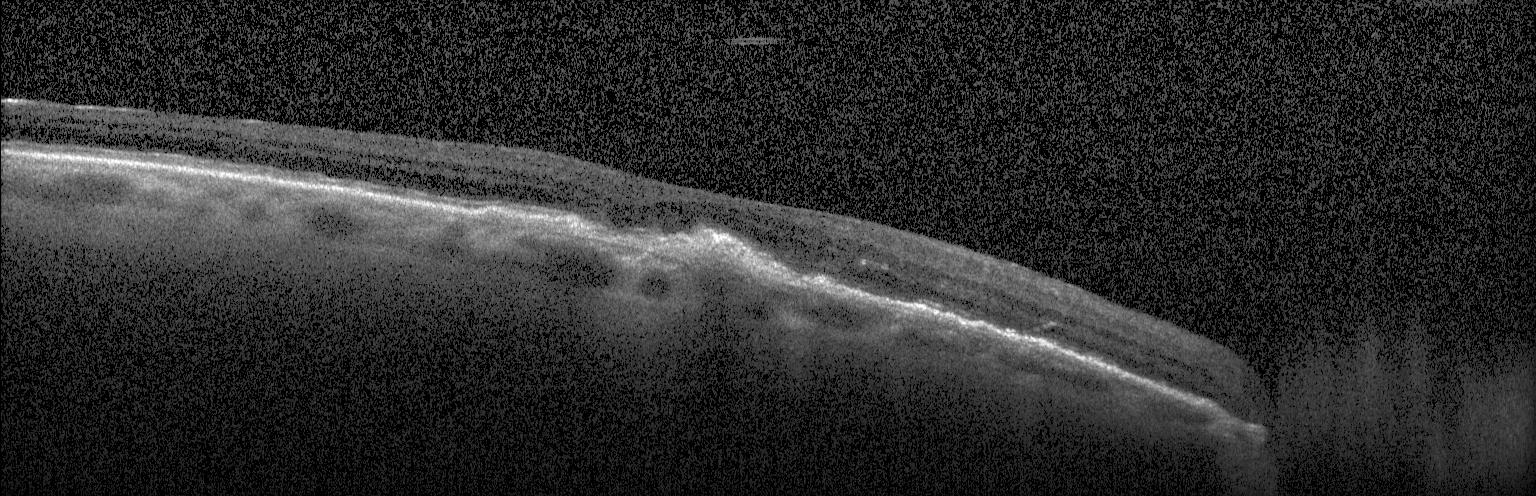 Choroidal neovascularization.